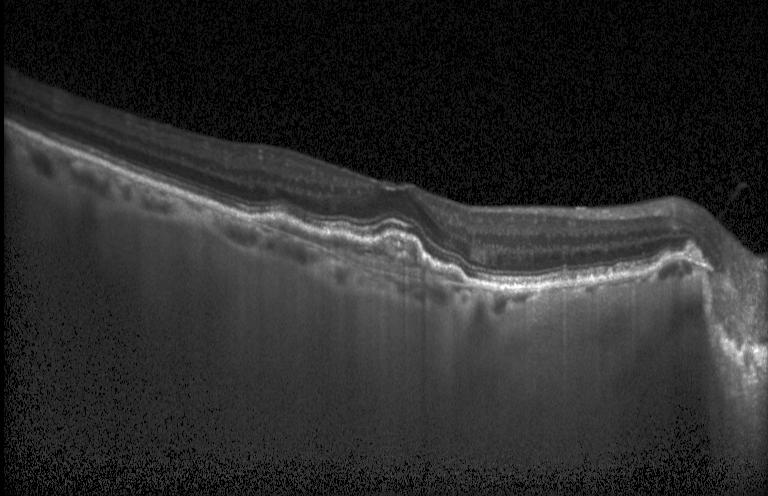
Optical coherence tomography scan; Heidelberg Spectralis.
Dx: CNV.